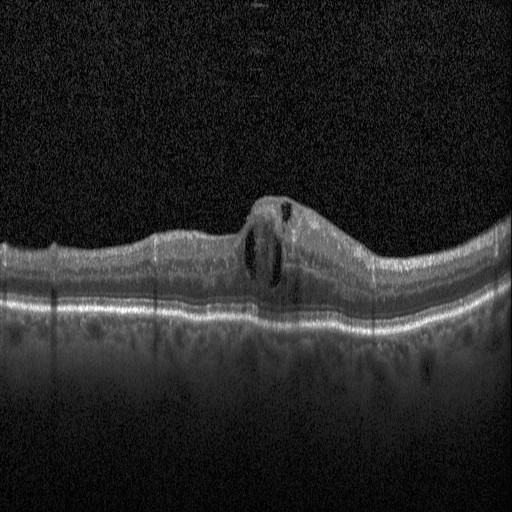
Optical coherence tomography B-scan; centered on the fovea — Diabetic macular edema (DME).